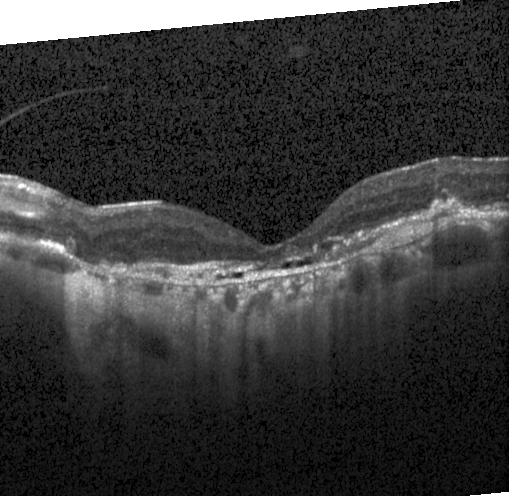

Diagnosis: CNV.